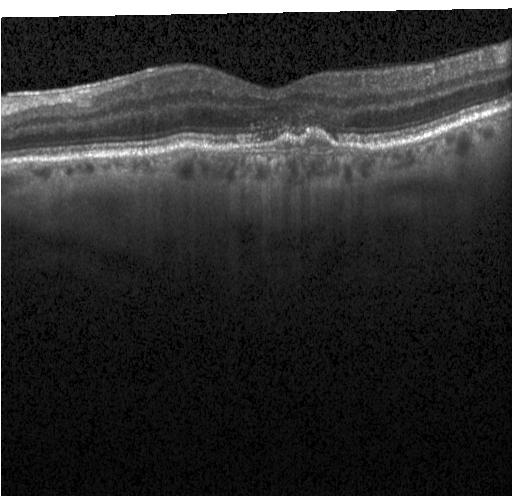
Optical coherence tomography B-scan
This B-scan demonstrates a choroidal neovascular membrane.